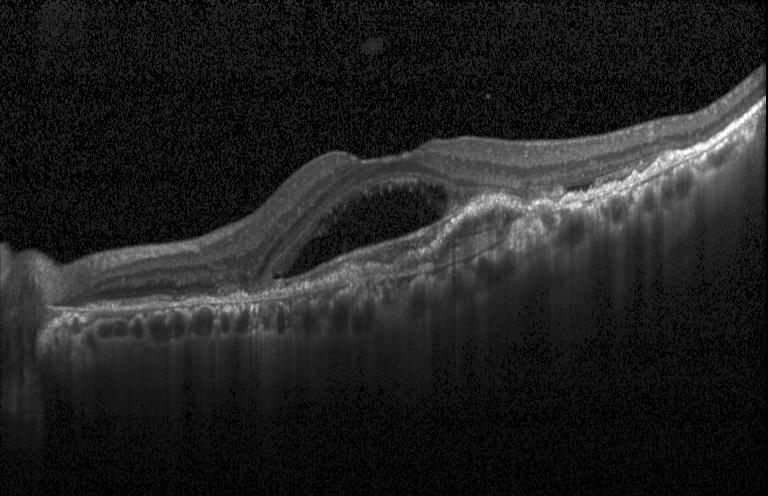
Dx: choroidal neovascularization.